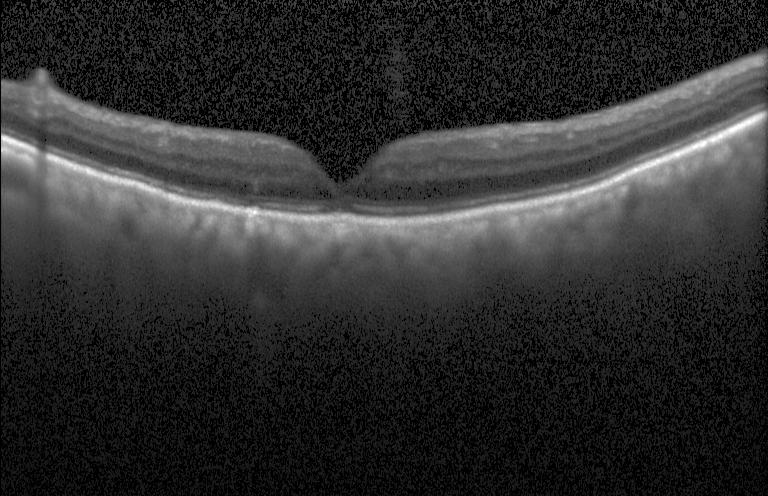 Impression: no evidence of choroidal neovascularization, diabetic macular edema, or drusen.